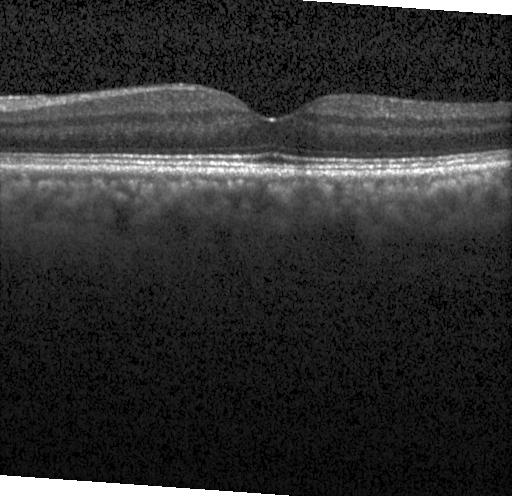

OCT line scan. Macular OCT: no choroidal neovascularization, diabetic macular edema, or drusen.